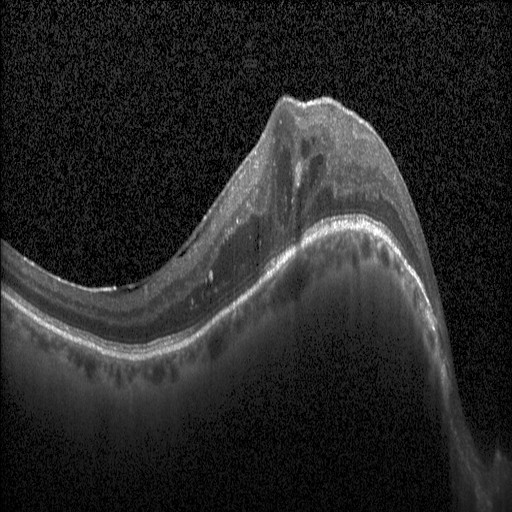

Optical coherence tomography scan — Diagnosis: diabetic macular edema (DME).